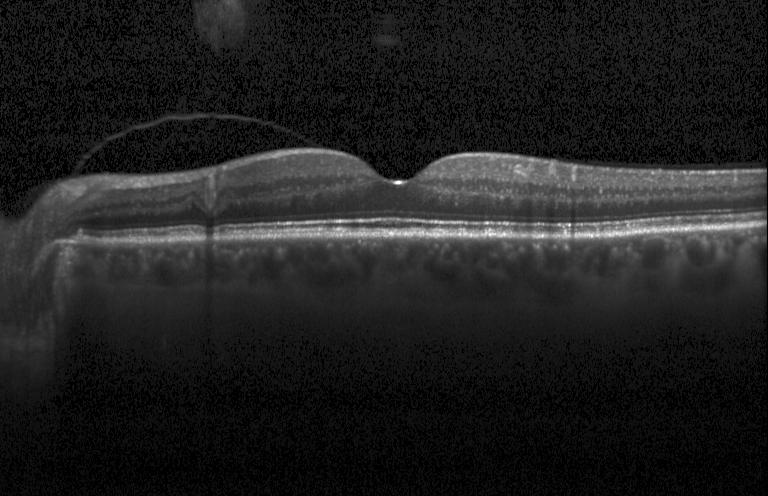
OCT B-scan · acquired on a Heidelberg Spectralis. Diagnosis: neither choroidal neovascularization, diabetic macular edema, nor drusen.